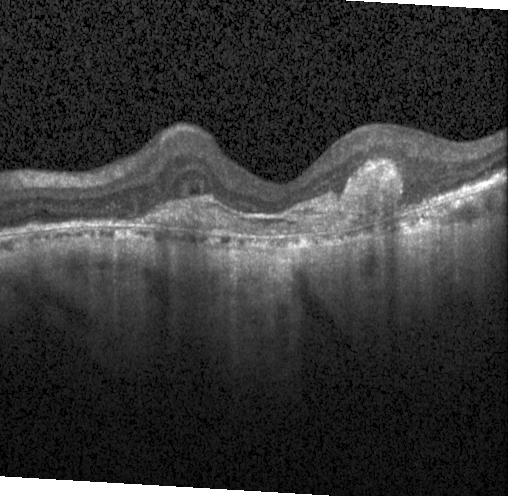

Retinal OCT cross-section, spectral-domain optical coherence tomography, through the macula
Finding: choroidal neovascularization (CNV).